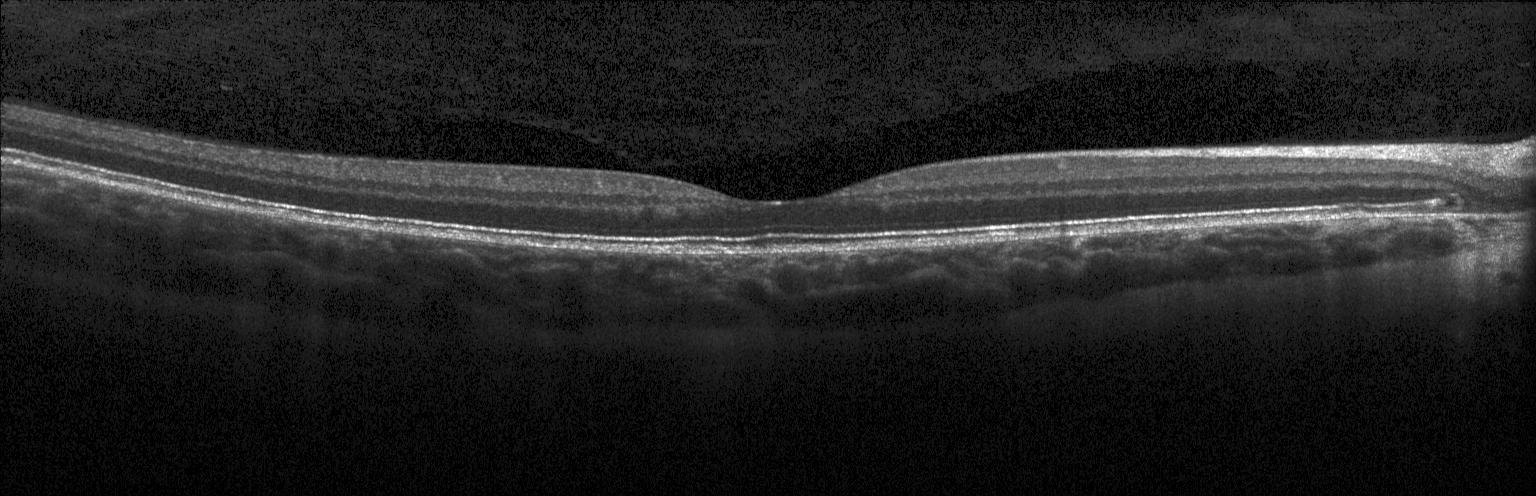
Retinal OCT B-scan, SD-OCT, centered on the fovea.
The scan shows no evidence of choroidal neovascularization, diabetic macular edema, or drusen.